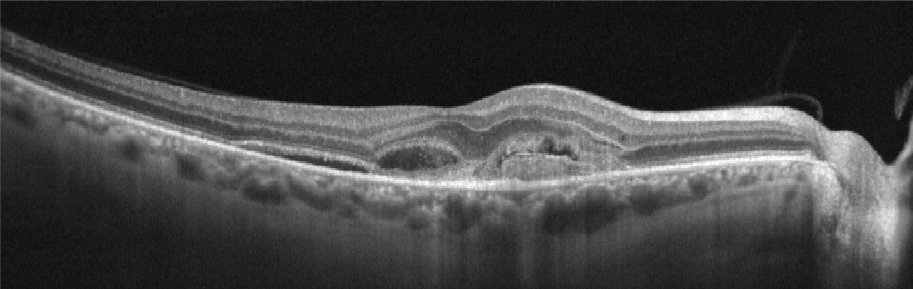 Retinal OCT B-scan. Impression: age-related macular degeneration (AMD).